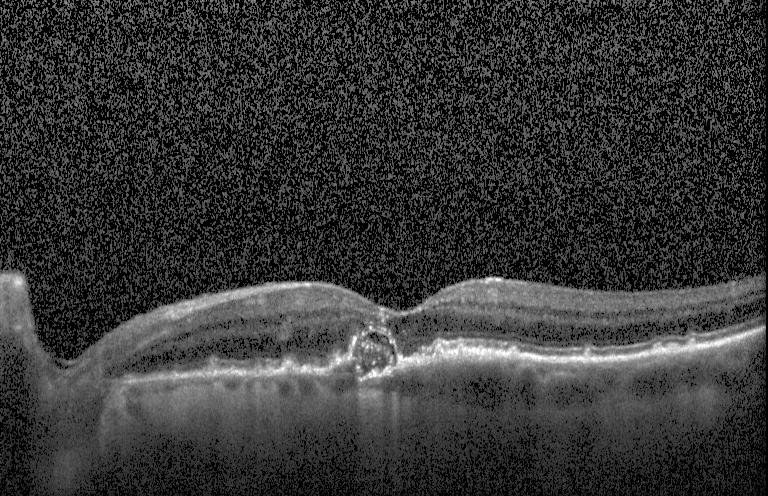
Centered on the fovea. Spectral-domain optical coherence tomography. Retinal OCT B-scan — The scan shows a choroidal neovascular membrane.